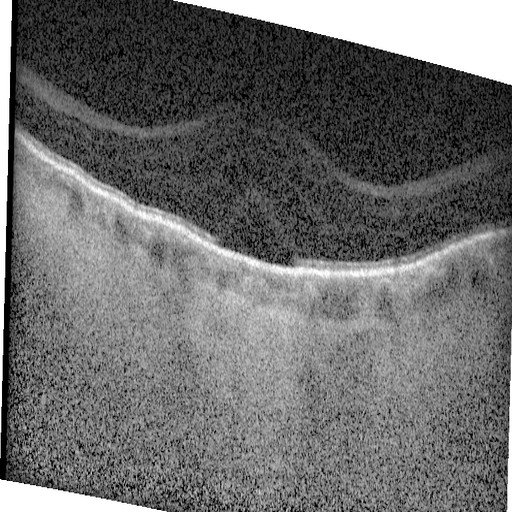

Retinal OCT cross-section. This B-scan demonstrates diabetic macular edema (DME).